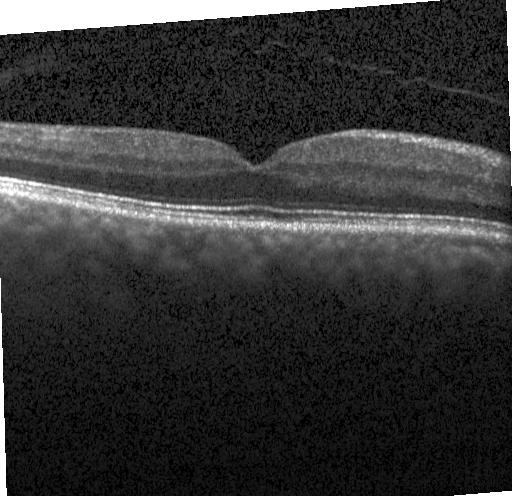
Impression: neither CNV, DME, nor drusen.